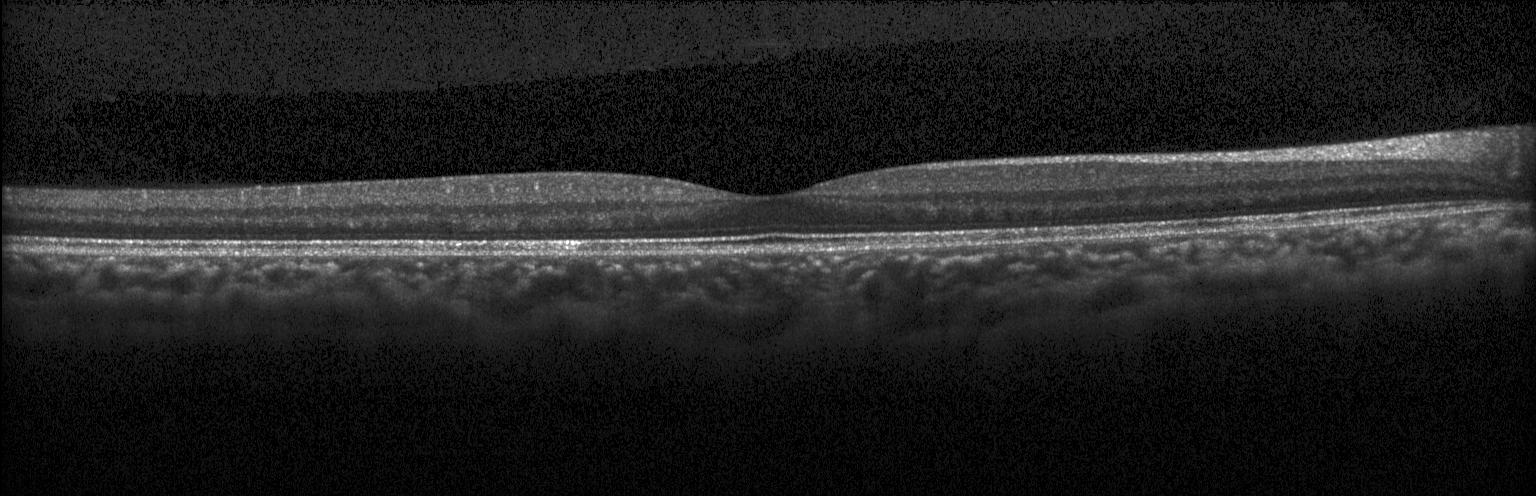
Retinal OCT cross-section
Dx: neither choroidal neovascularization, diabetic macular edema, nor drusen.